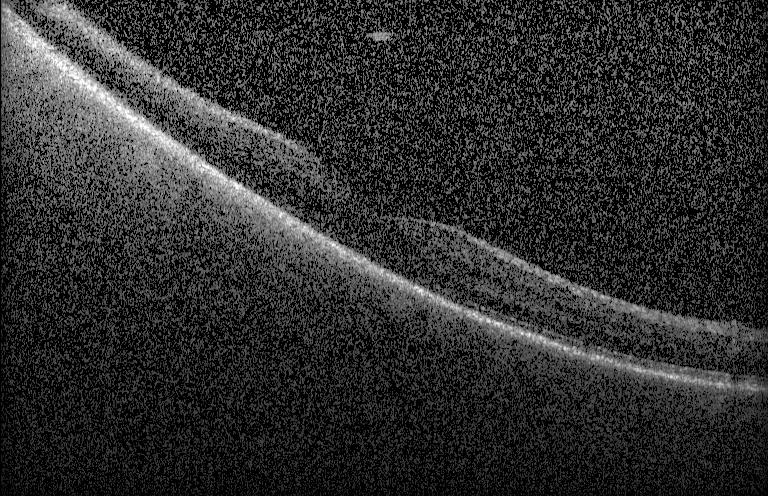
Spectral-domain OCT · optical coherence tomography B-scan · Heidelberg Spectralis OCT system · horizontal scan through the fovea. Finding: no CNV, no DME, and no drusen.